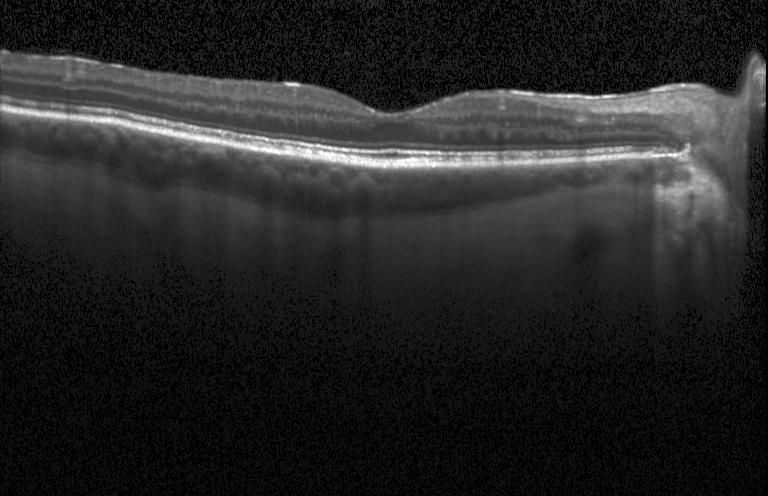
Spectral-domain OCT. Optical coherence tomography scan. Through the macula.
Diagnosis: no choroidal neovascularization, no diabetic macular edema, and no drusen.